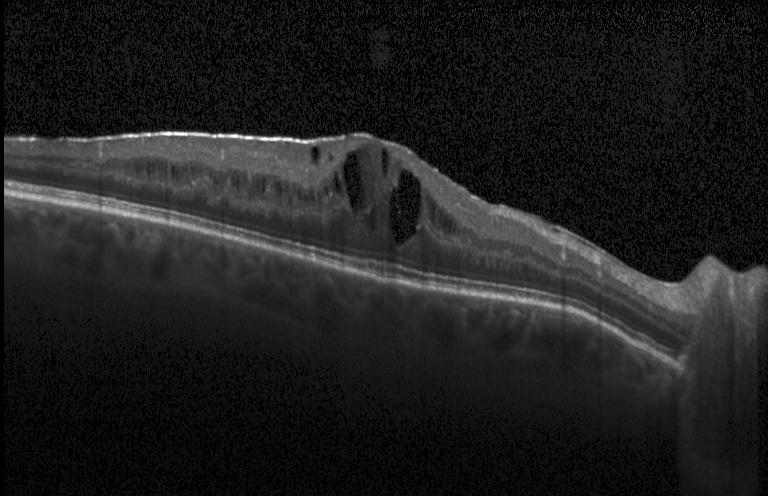
Instrument: Heidelberg Spectralis, optical coherence tomography B-scan, through the macula, spectral-domain OCT — Macular OCT: DME.